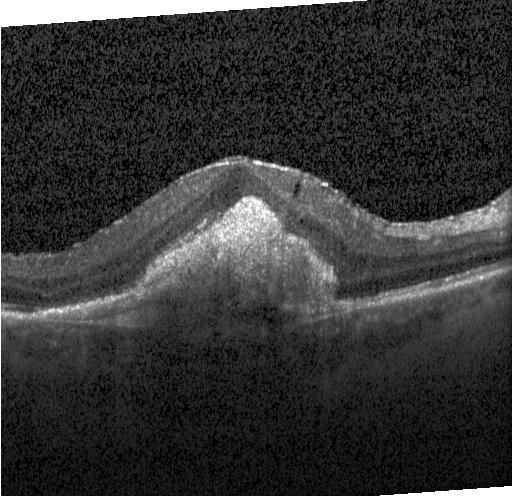 Impression: choroidal neovascularization (CNV).